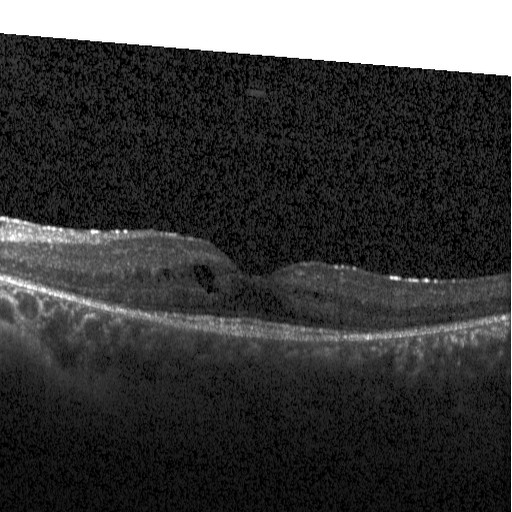
SD-OCT. Retinal OCT cross-section. Heidelberg Spectralis OCT system. OCT finding: diabetic macular edema (DME).